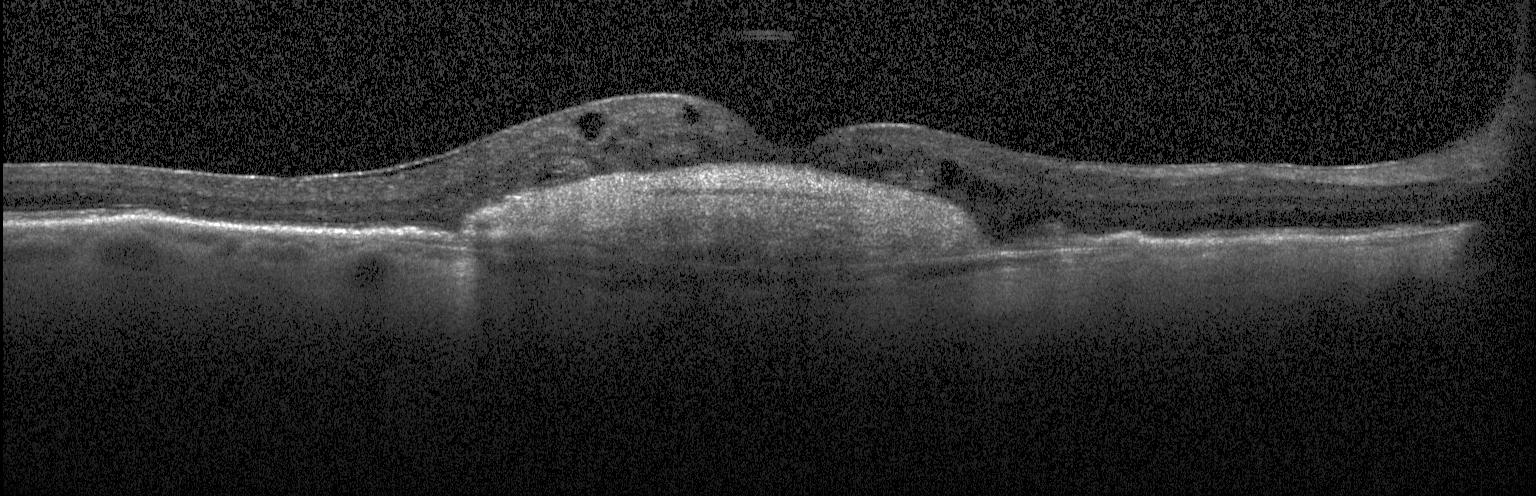 Heidelberg Spectralis OCT system · OCT B-scan. The scan shows a choroidal neovascular membrane.